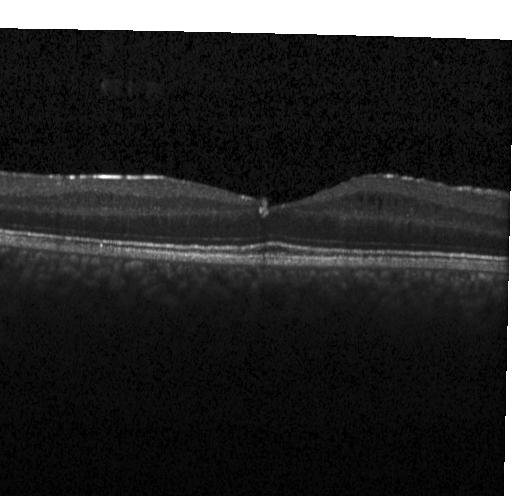

Optical coherence tomography scan · SD-OCT · instrument: Heidelberg Spectralis. Assessment: diabetic macular edema (DME).